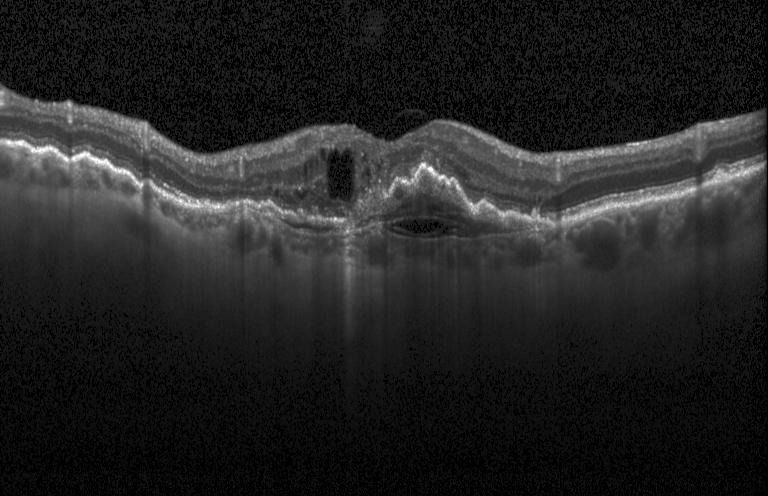
Dx: a choroidal neovascular membrane.